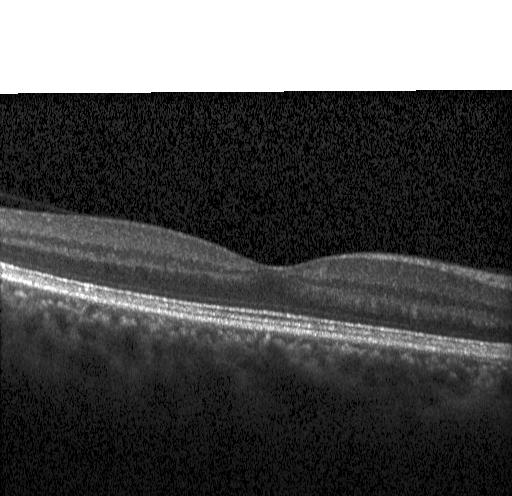 Acquired on a Heidelberg Spectralis, retinal OCT cross-section, SD-OCT — Impression: no CNV, DME, or drusen.